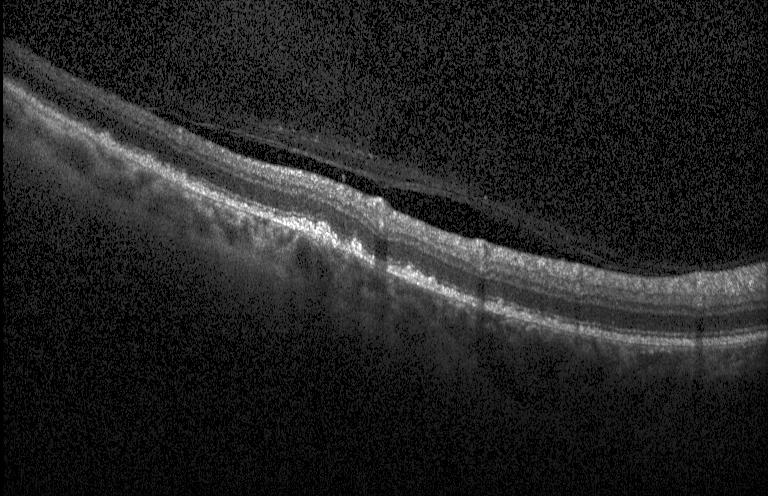
Optical coherence tomography B-scan · acquired on a Heidelberg Spectralis
Finding: sub-RPE drusenoid deposits.